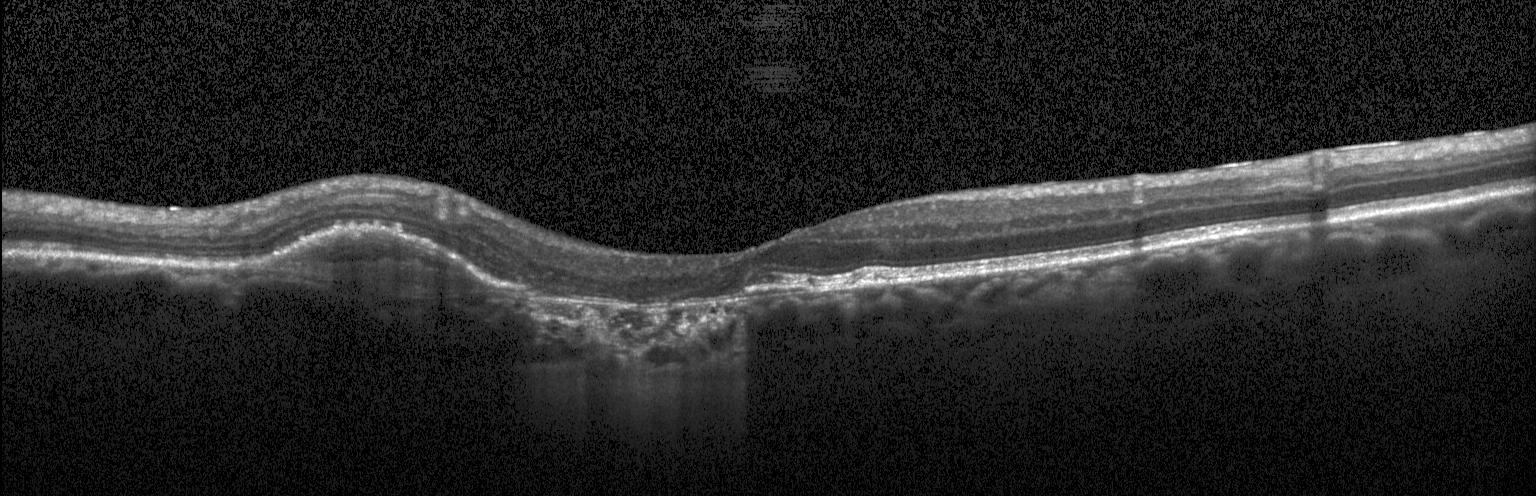
Retinal OCT cross-section. Instrument: Heidelberg Spectralis. Horizontal scan through the fovea.
Finding: choroidal neovascularization (CNV).